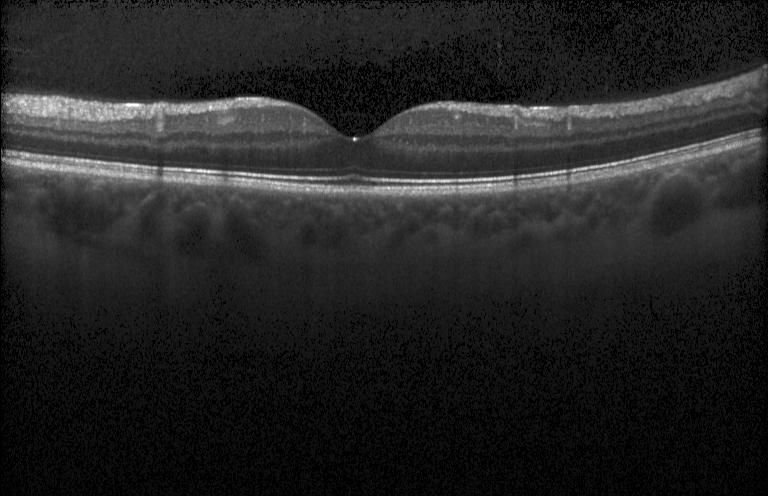
Diagnosis: no CNV, no DME, and no drusen.